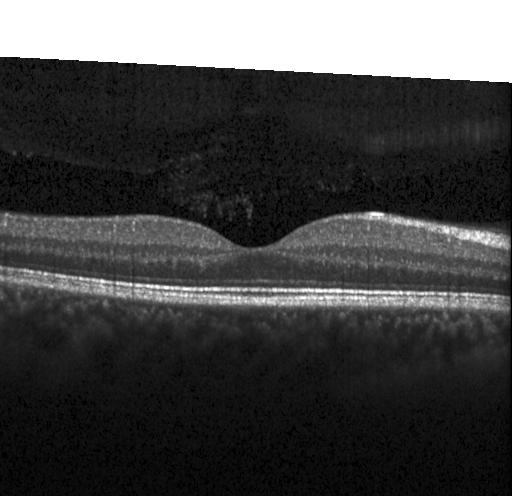
Finding: neither choroidal neovascularization, diabetic macular edema, nor drusen.